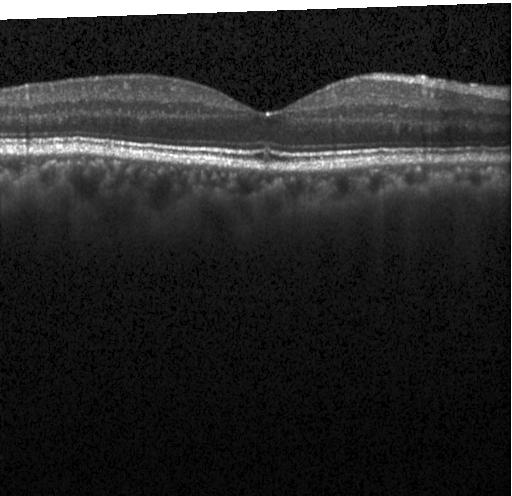 Spectral-domain OCT B-scan: no choroidal neovascularization, diabetic macular edema, or drusen.